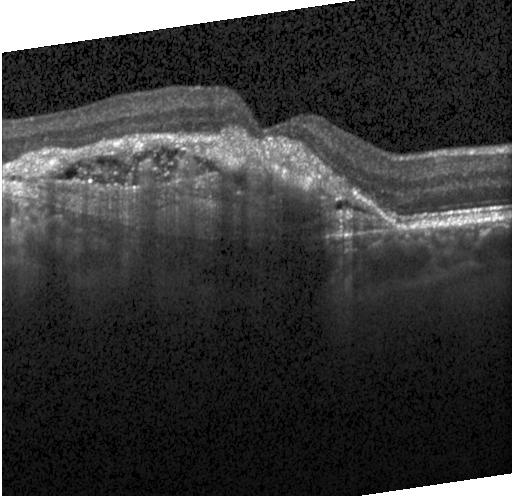

Diagnosis: a choroidal neovascular membrane.